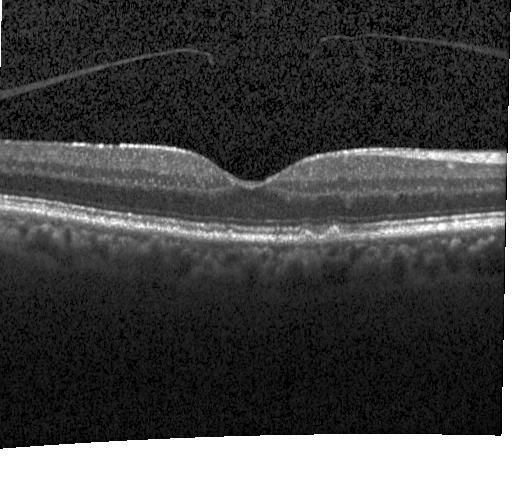 Macular OCT demonstrating sub-RPE drusenoid deposits.